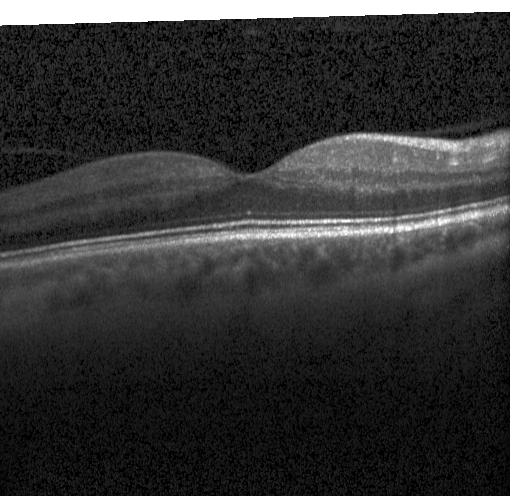 Optical coherence tomography scan; through the macula; Heidelberg Spectralis OCT system.
Impression: no CNV, no DME, and no drusen.